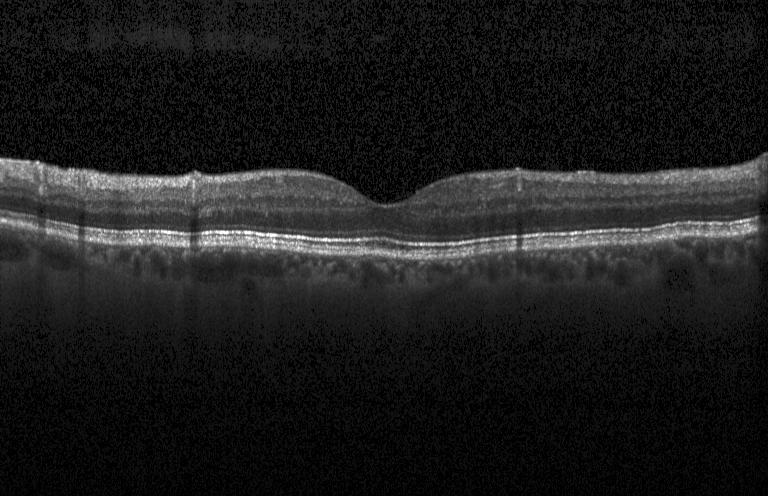 OCT B-scan showing no CNV, DME, or drusen.